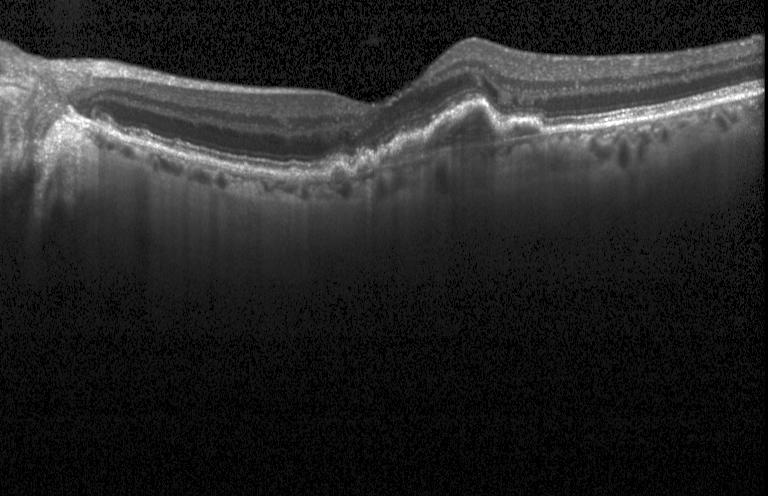

SD-OCT. Centered on the fovea. Acquired on a Heidelberg Spectralis. Optical coherence tomography B-scan. Diagnosis: CNV.